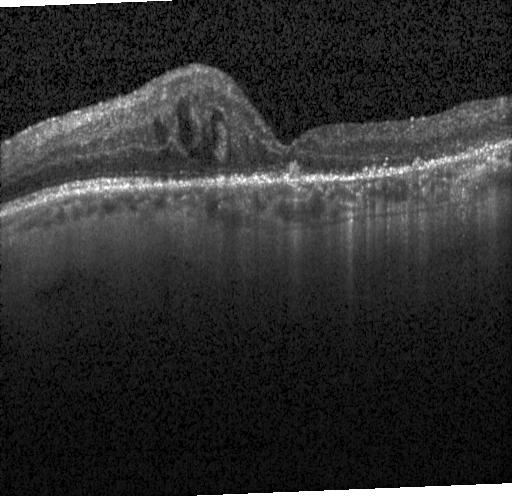 OCT line scan; through the macula. Impression: diabetic macular edema (DME).